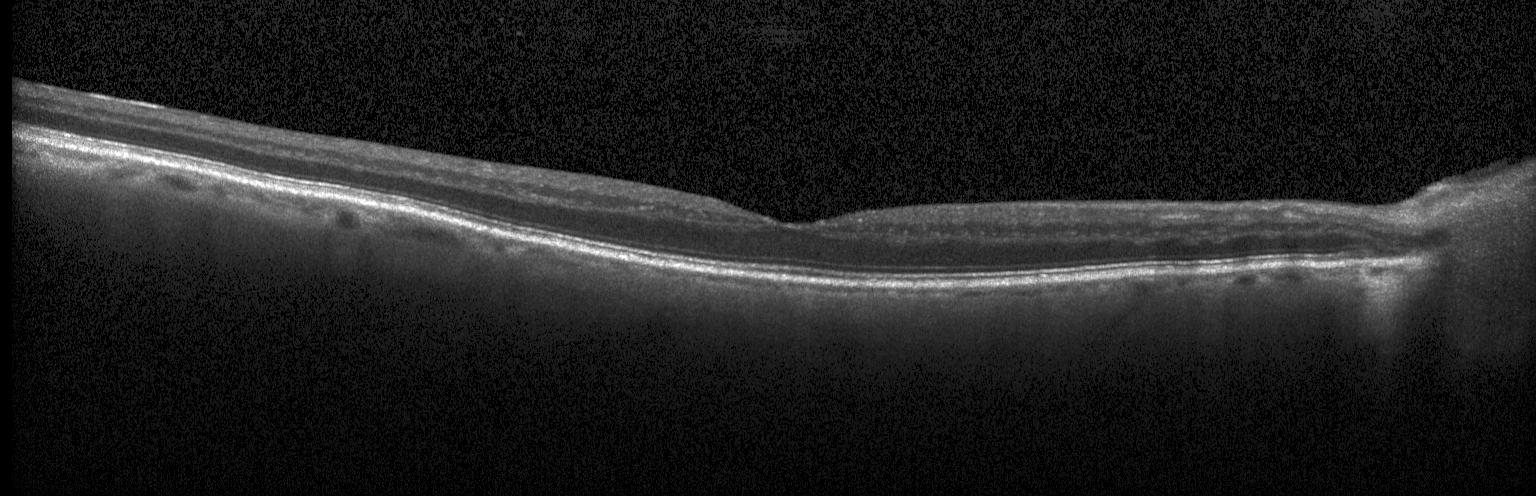 Macular OCT: no evidence of choroidal neovascularization, diabetic macular edema, or drusen.